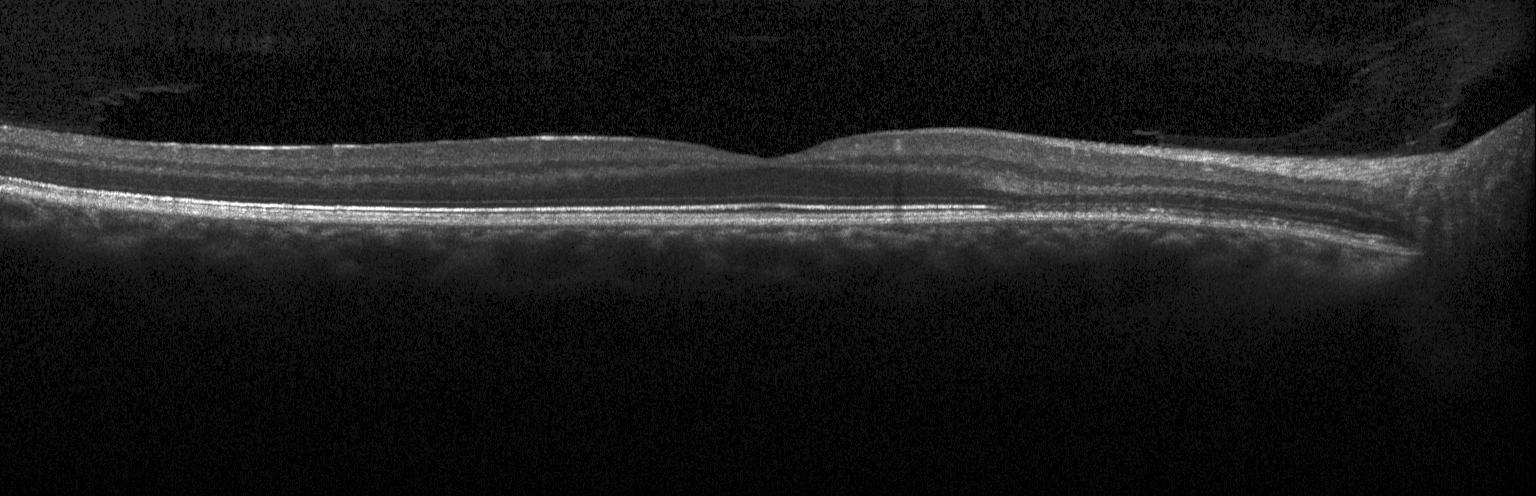

Retinal OCT cross-section.
Impression: no evidence of choroidal neovascularization, diabetic macular edema, or drusen.